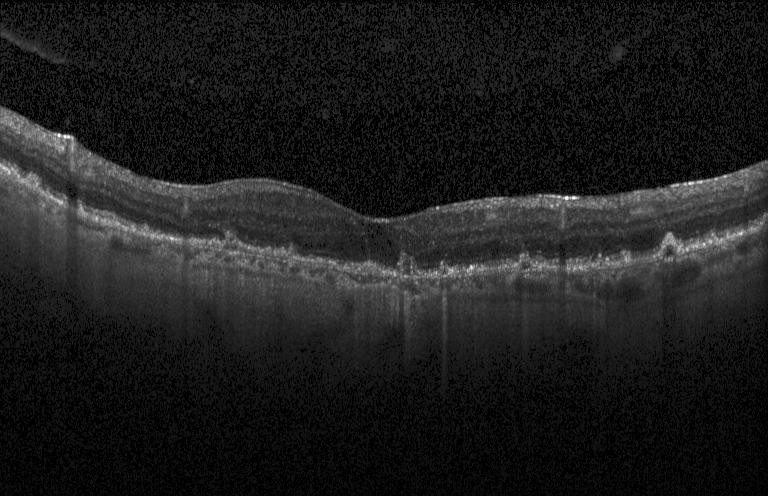
Optical coherence tomography B-scan. Spectral-domain optical coherence tomography.
Dx: choroidal neovascularization (CNV).